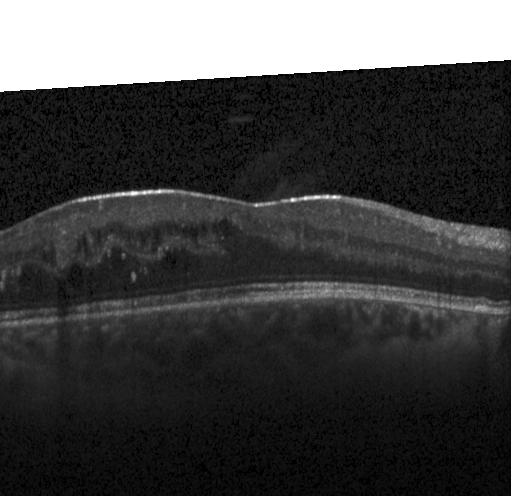

Diagnosis: diabetic macular edema.